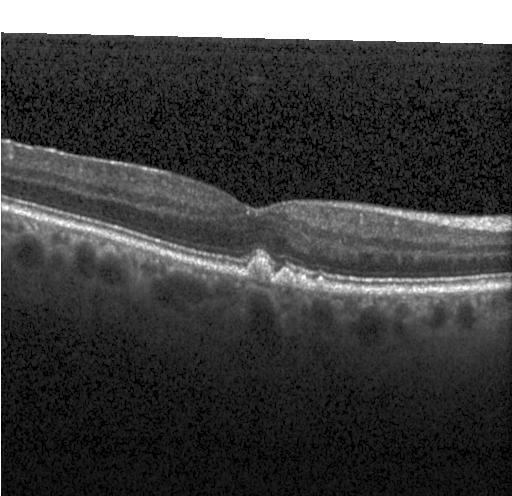 Macular OCT demonstrating multiple drusen.